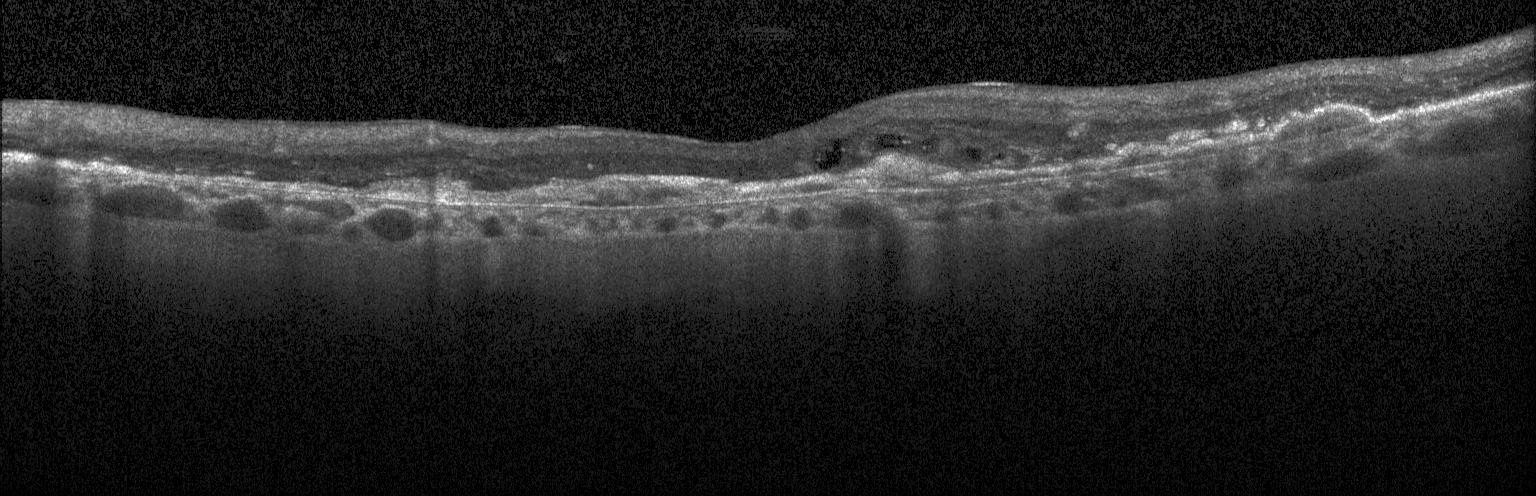
Diagnosis: a choroidal neovascular membrane.